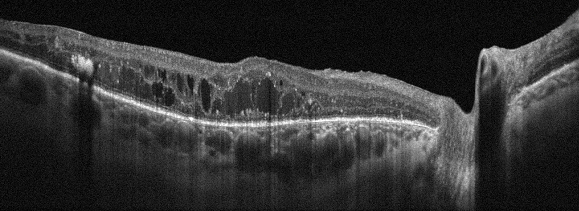
Optical coherence tomography B-scan, instrument: Optovue Avanti RTVue XR, fovea-centered — The scan shows DME.